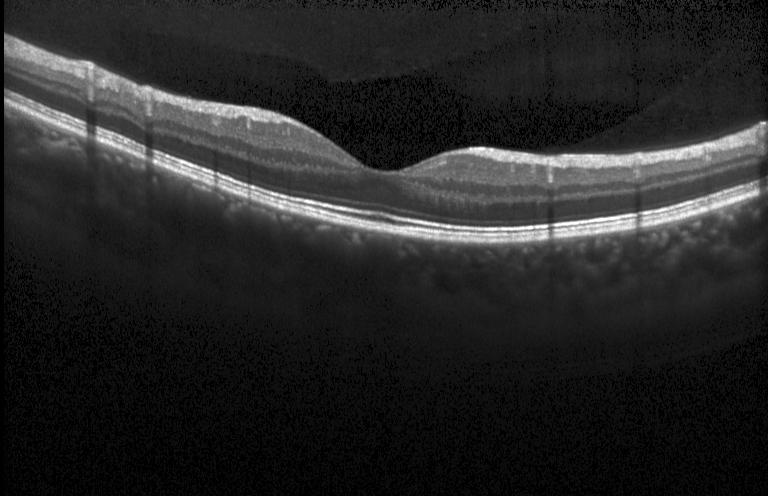
Macular OCT demonstrating no choroidal neovascularization, diabetic macular edema, or drusen.